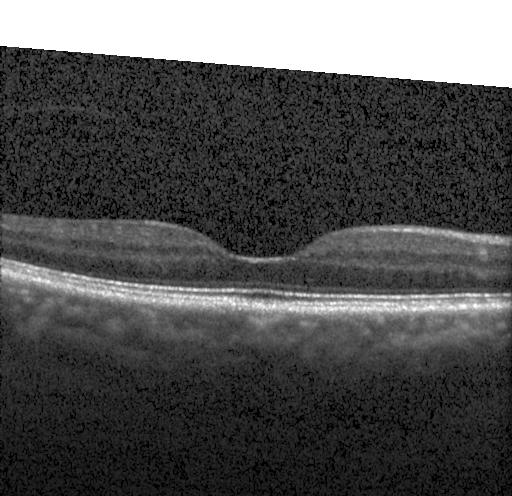

OCT finding: no CNV, no DME, and no drusen.